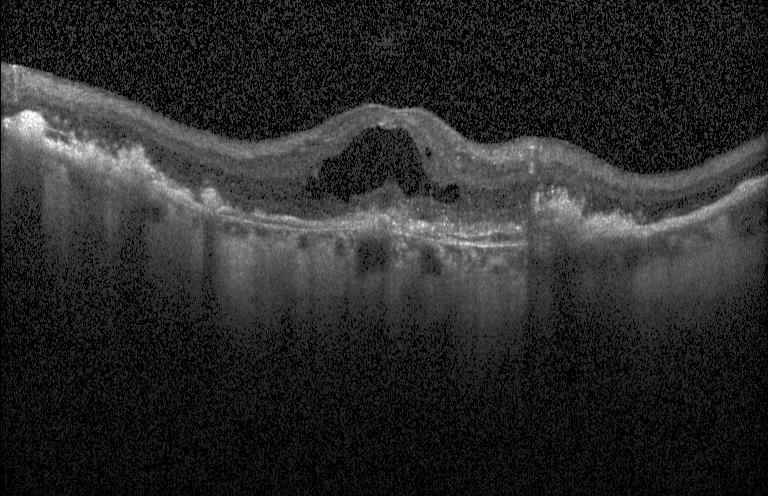
Spectral-domain OCT B-scan: choroidal neovascularization (CNV).